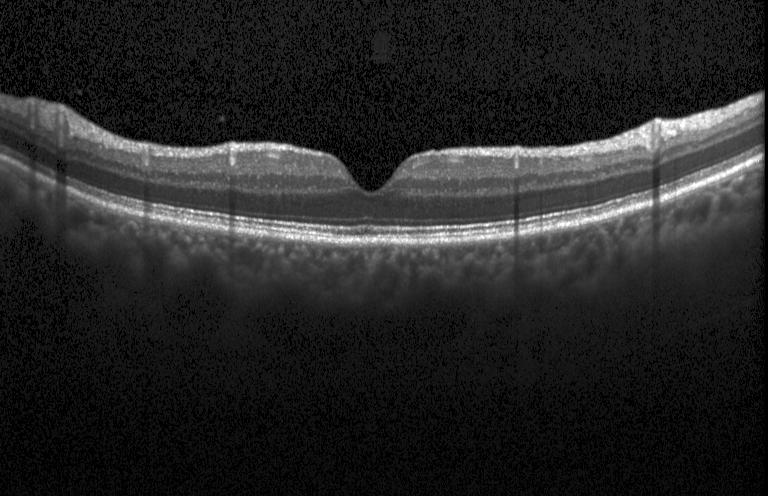 Through the macula; OCT line scan; spectral-domain OCT. Finding: no evidence of choroidal neovascularization, diabetic macular edema, or drusen.